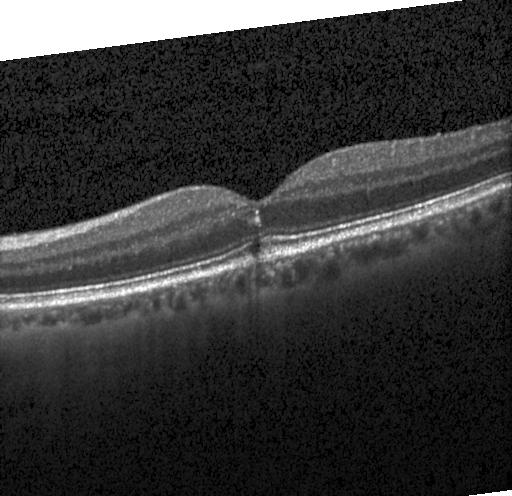 OCT finding: choroidal neovascularization.